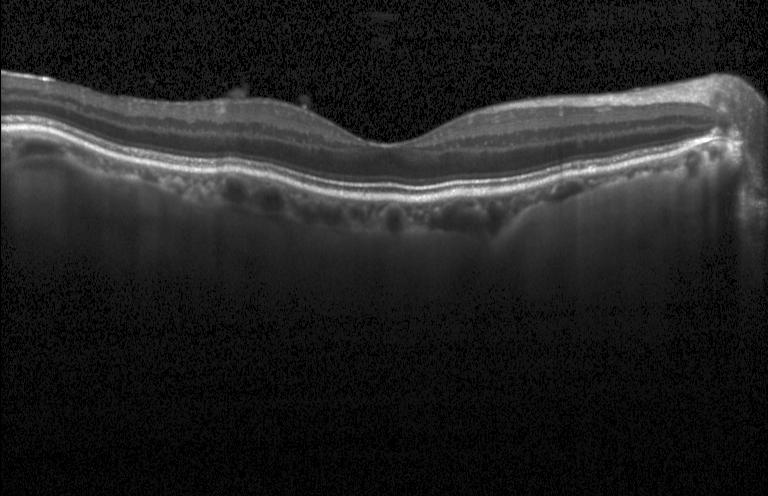
Spectral-domain optical coherence tomography · retinal OCT B-scan · horizontal scan through the fovea · acquired on a Heidelberg Spectralis — Finding: no evidence of choroidal neovascularization, diabetic macular edema, or drusen.